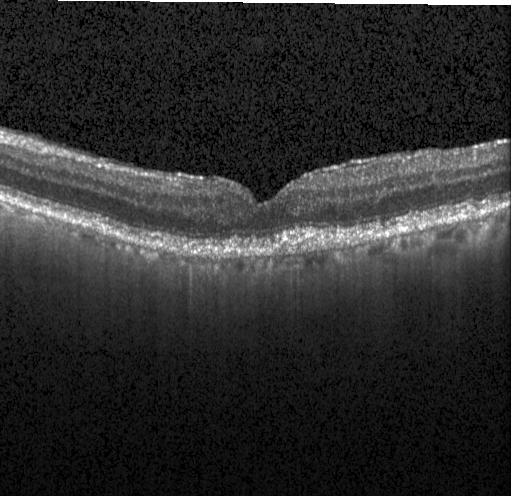 Diagnosis: sub-RPE drusenoid deposits.